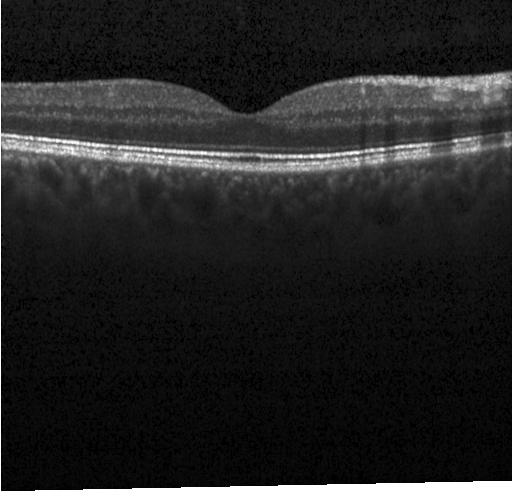
Retinal OCT cross-section — Impression: no CNV, DME, or drusen.